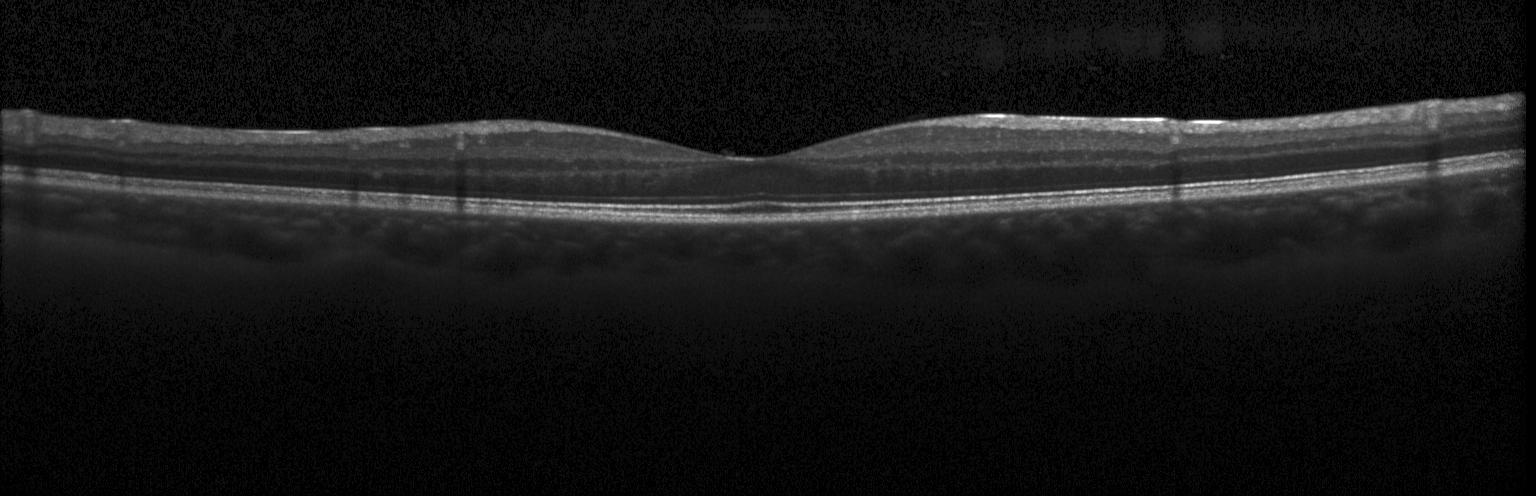

Finding: neither CNV, DME, nor drusen.